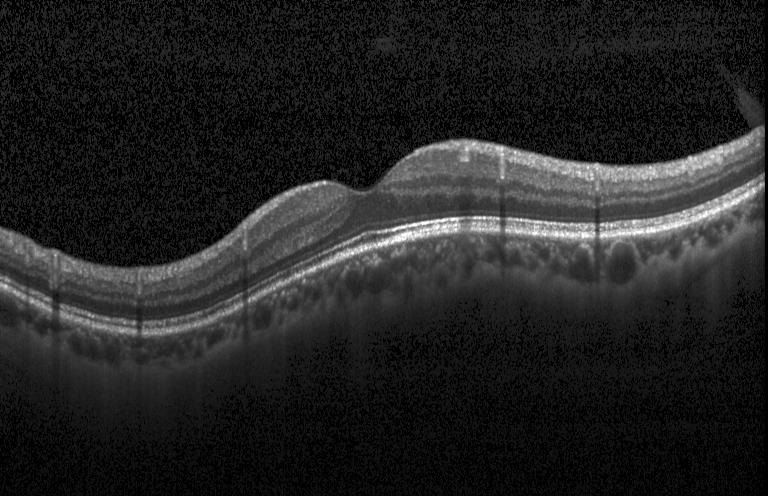

Spectral-domain OCT; optical coherence tomography B-scan.
Dx: no evidence of choroidal neovascularization, diabetic macular edema, or drusen.